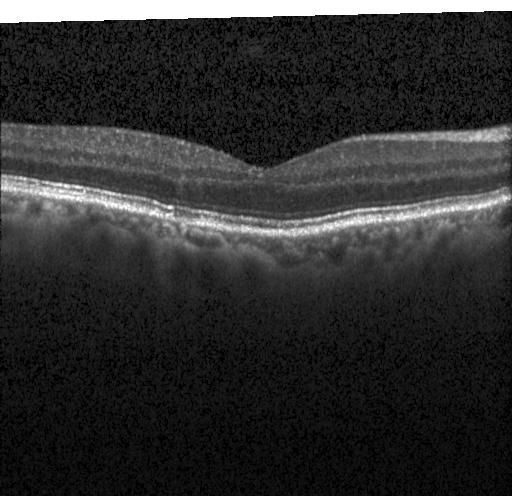 OCT line scan, spectral-domain OCT.
Impression: no evidence of choroidal neovascularization, diabetic macular edema, or drusen.